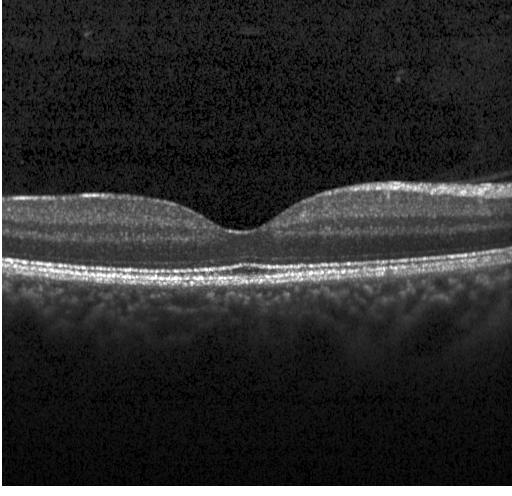

Optical coherence tomography scan.
Assessment: neither choroidal neovascularization, diabetic macular edema, nor drusen.